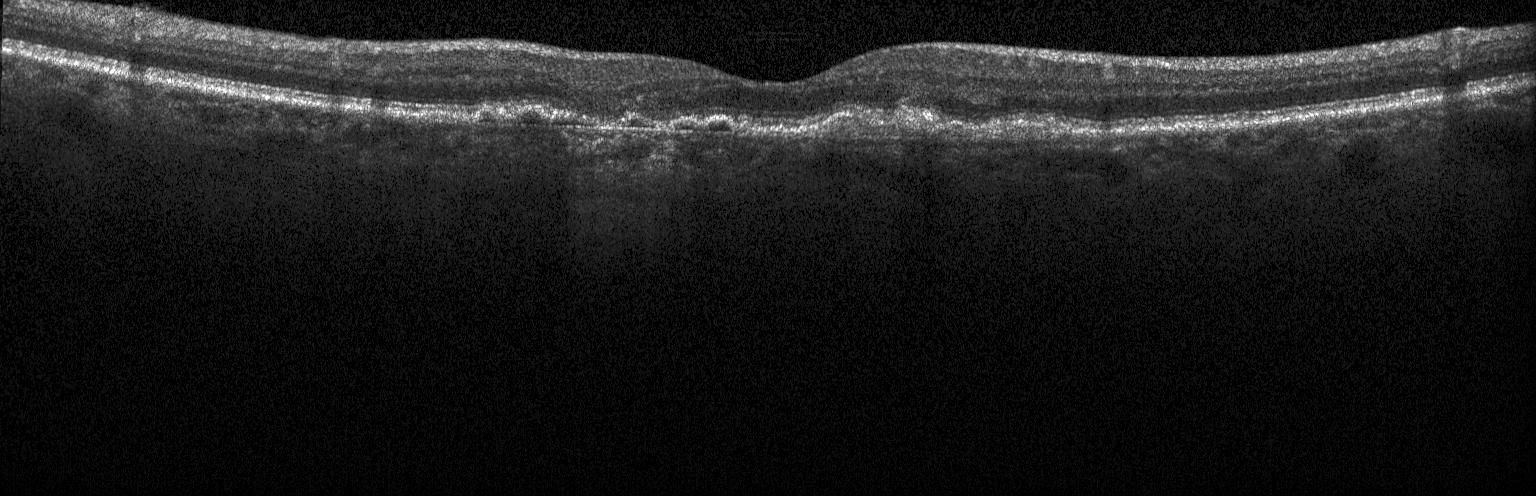
Retinal OCT cross-section.
Diagnosis: a choroidal neovascular membrane.